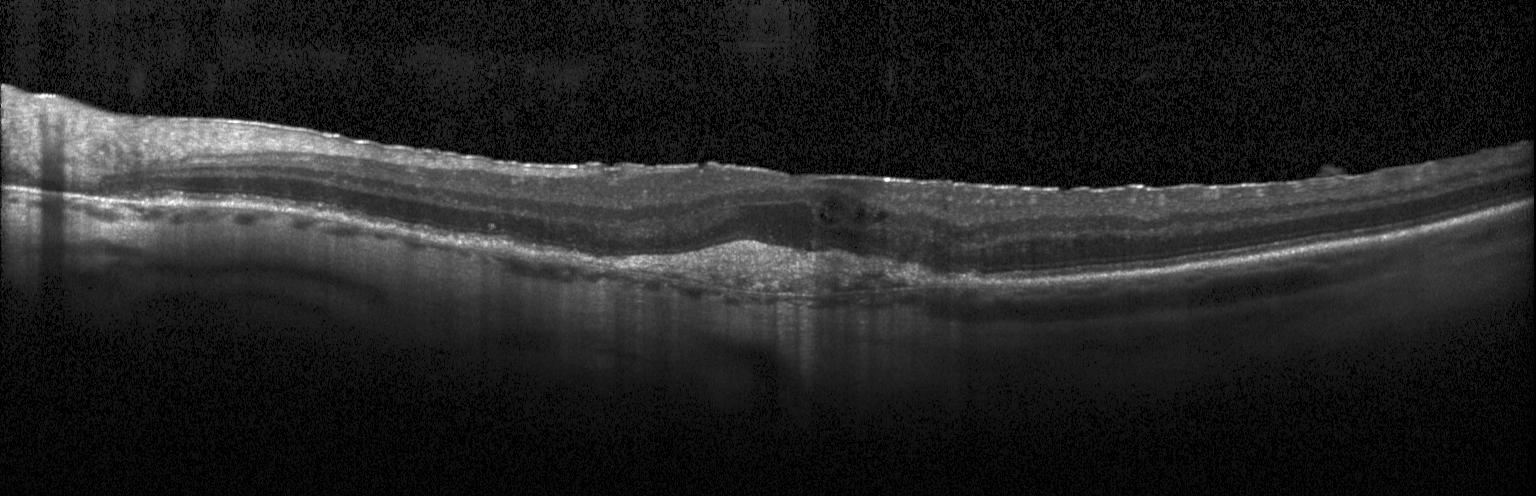

Centered on the fovea. Retinal OCT cross-section — Choroidal neovascularization.